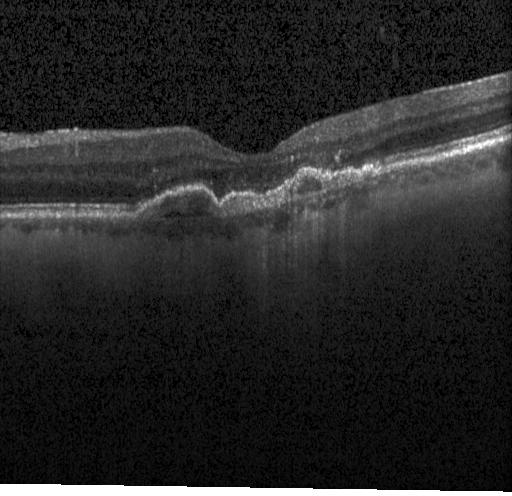
Finding: choroidal neovascularization.